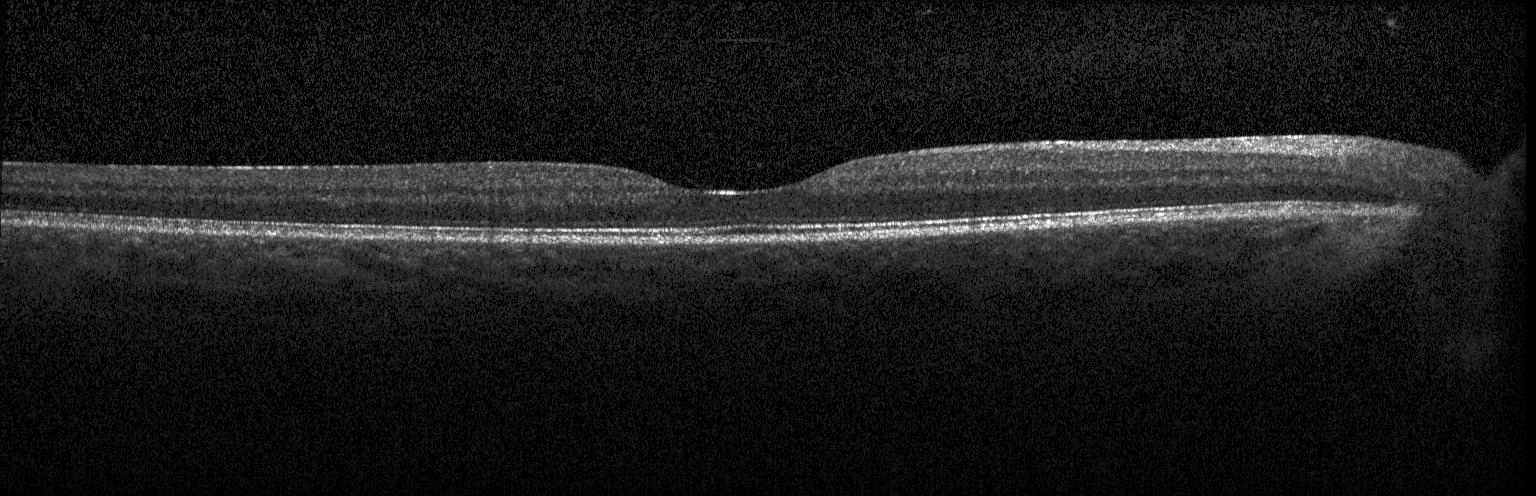 The scan shows no CNV, DME, or drusen.